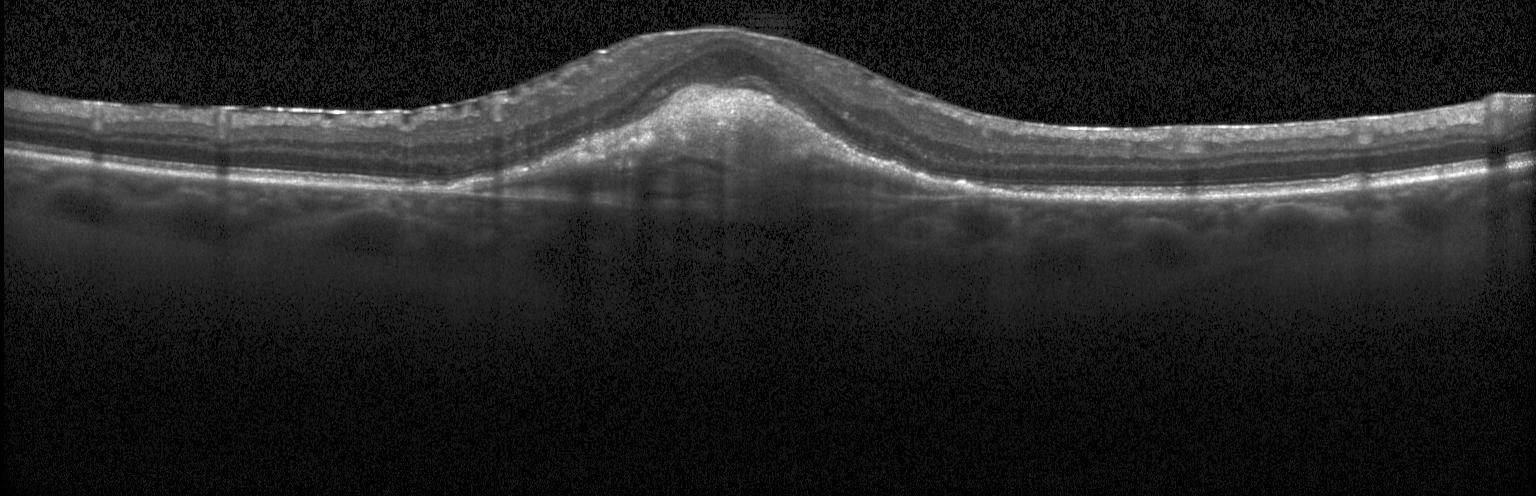 Horizontal scan through the fovea, instrument: Heidelberg Spectralis, retinal OCT B-scan. Impression: CNV.